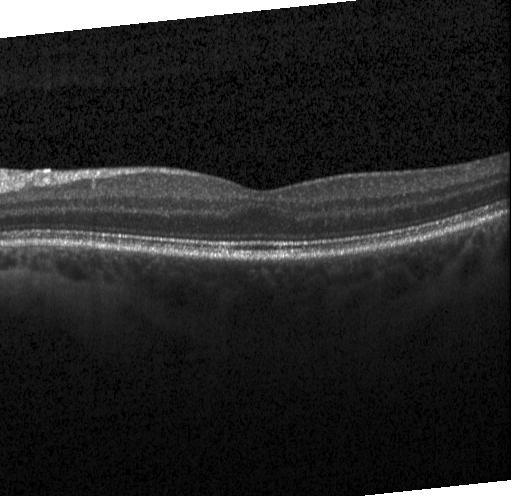 OCT B-scan · Heidelberg Spectralis OCT system.
Diagnosis: no evidence of CNV, DME, or drusen.